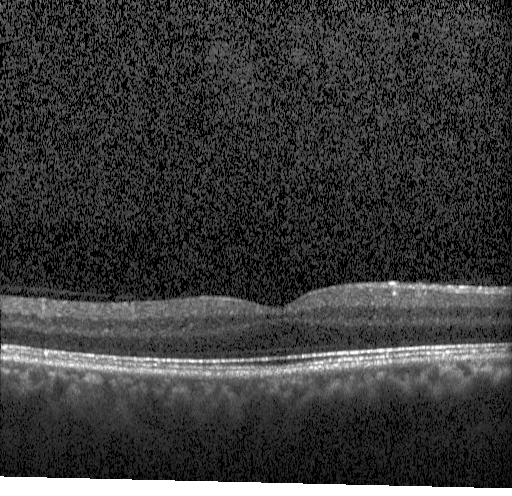
Retinal OCT B-scan
Dx: neither choroidal neovascularization, diabetic macular edema, nor drusen.